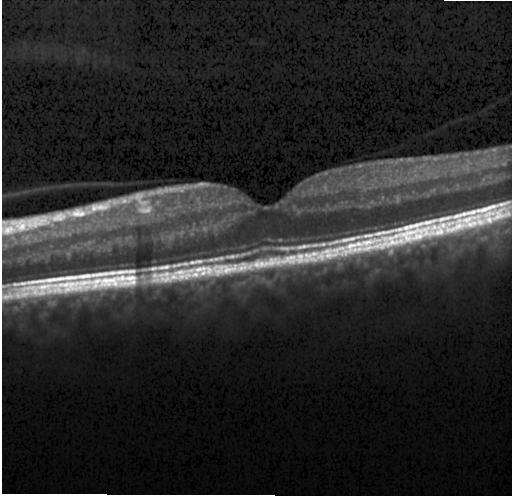
Finding: no choroidal neovascularization, no diabetic macular edema, and no drusen.